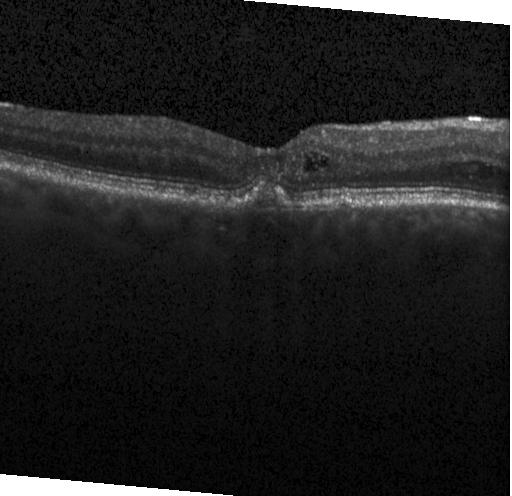 Spectral-domain optical coherence tomography. Optical coherence tomography B-scan. Centered on the fovea. Heidelberg Spectralis — Impression: a choroidal neovascular membrane.